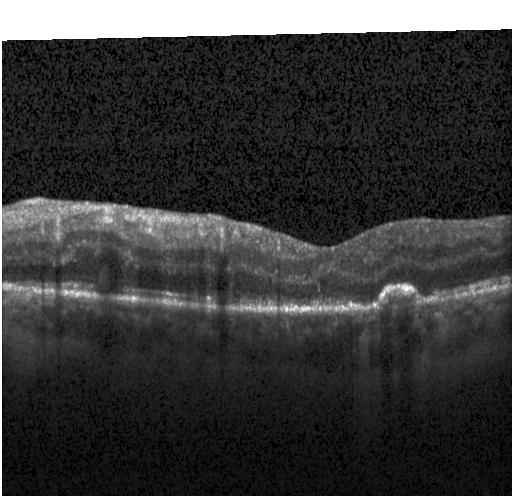

Dx: choroidal neovascularization.